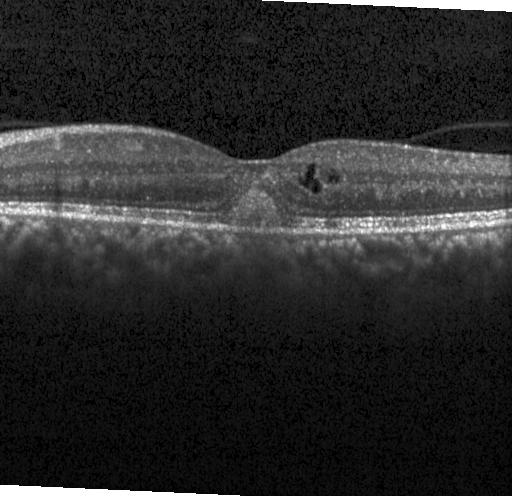
Retinal OCT B-scan
OCT finding: choroidal neovascularization (CNV).